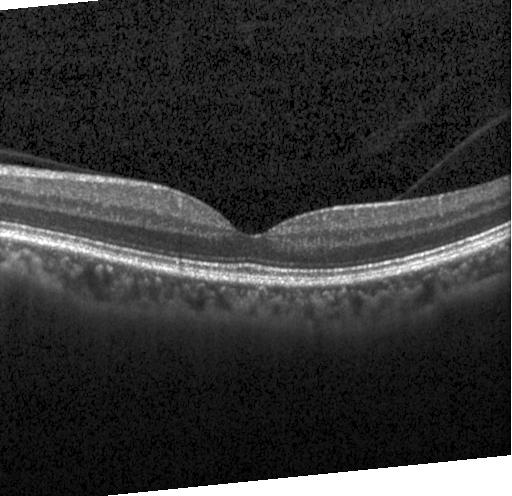

Heidelberg Spectralis. Optical coherence tomography scan. Finding: no CNV, DME, or drusen.